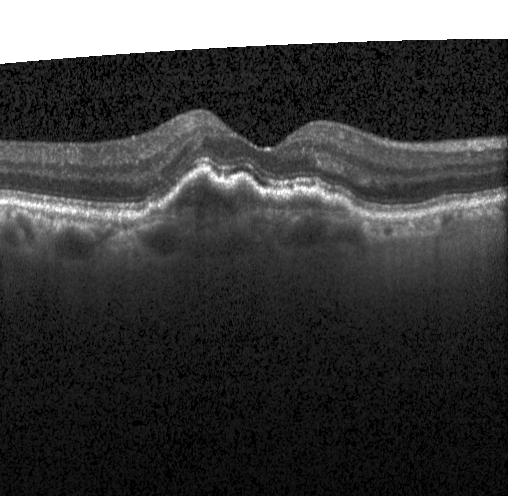

The scan shows choroidal neovascularization.